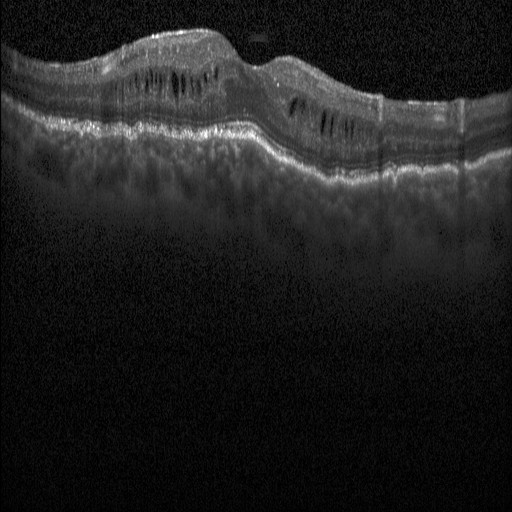 Macular OCT demonstrating diabetic macular edema.